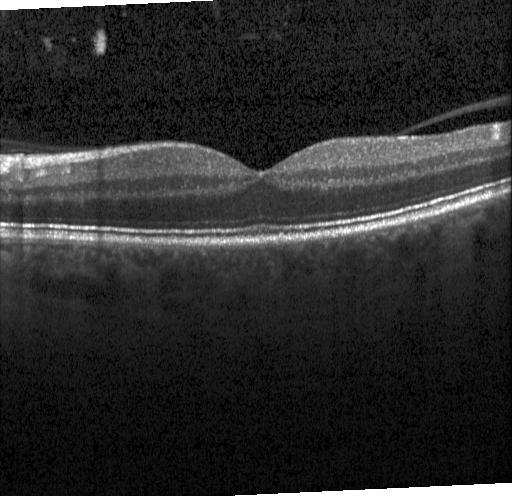 Horizontal scan through the fovea; spectral-domain optical coherence tomography; Heidelberg Spectralis OCT system; retinal OCT B-scan — Impression: neither choroidal neovascularization, diabetic macular edema, nor drusen.